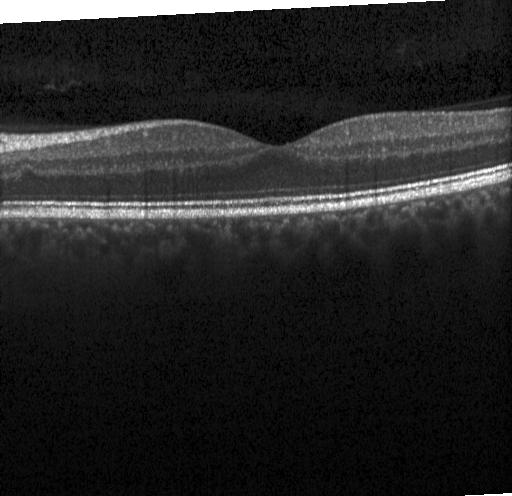
This B-scan demonstrates no choroidal neovascularization, diabetic macular edema, or drusen.